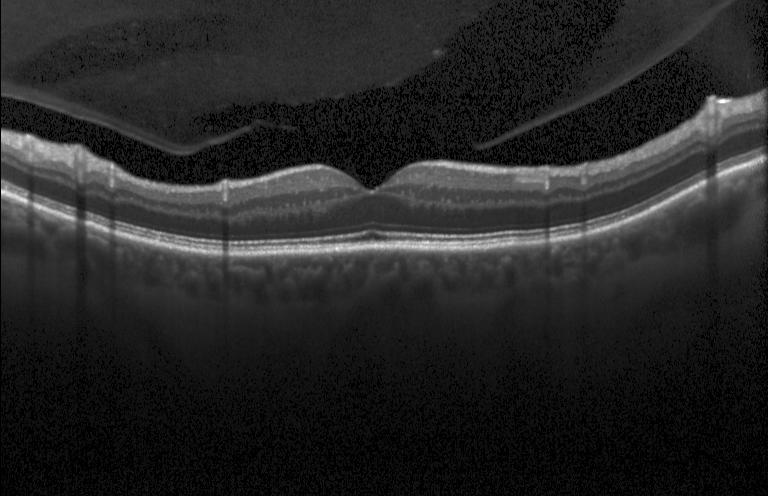 OCT scan showing neither CNV, DME, nor drusen.